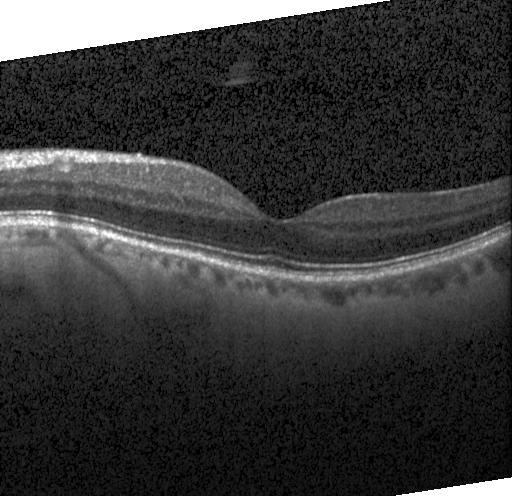 Dx: neither CNV, DME, nor drusen.